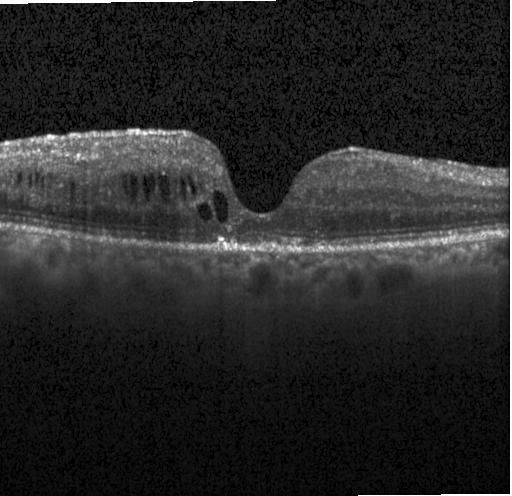
Acquired on a Heidelberg Spectralis, through the macula, OCT line scan — Diabetic macular edema.